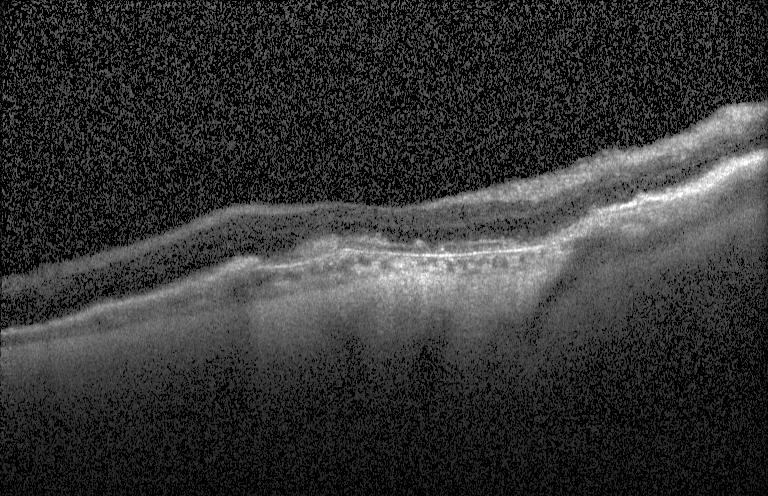
Retinal OCT B-scan.
This B-scan demonstrates choroidal neovascularization.